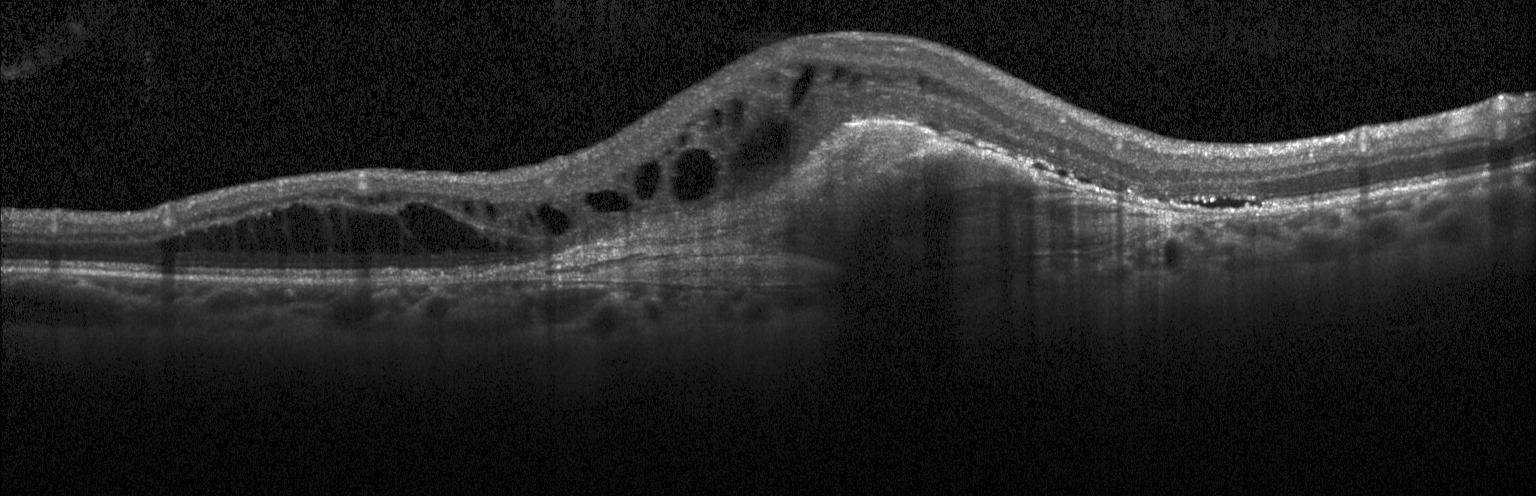 Retinal OCT cross-section showing a choroidal neovascular membrane.